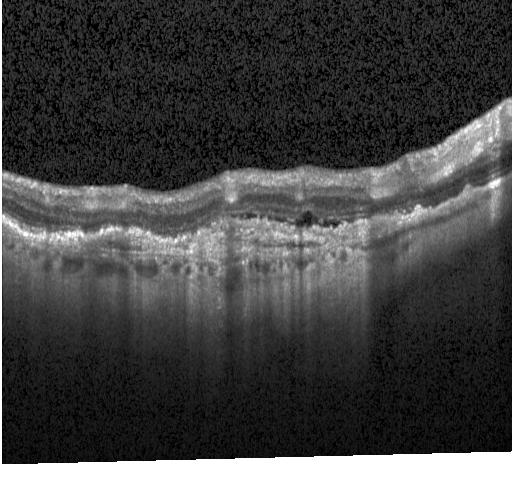 OCT finding: a choroidal neovascular membrane.